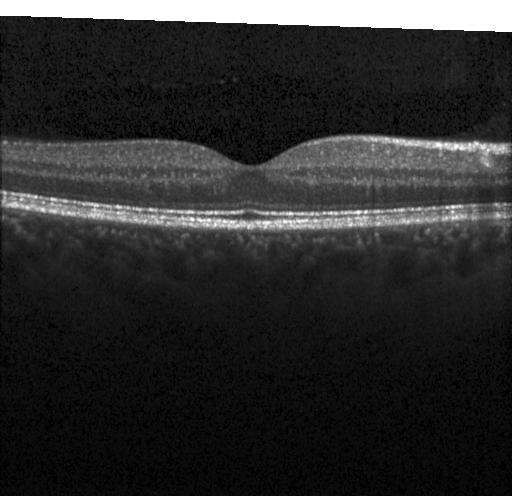
OCT line scan.
Assessment: no choroidal neovascularization, diabetic macular edema, or drusen.